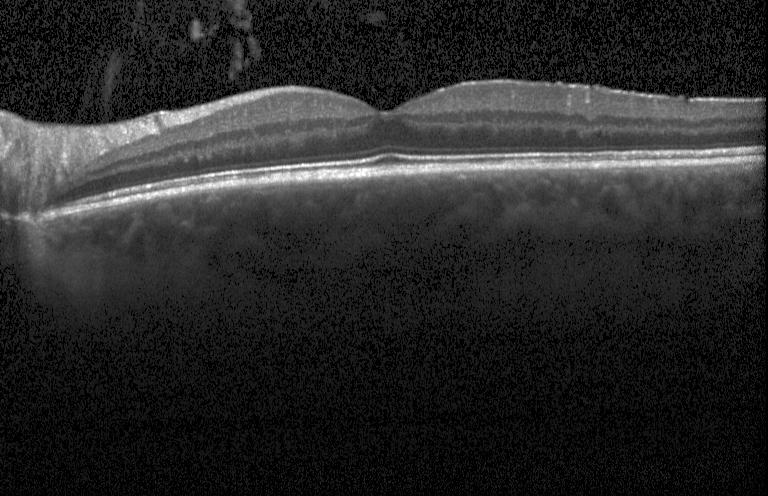 Optical coherence tomography B-scan — Dx: no evidence of choroidal neovascularization, diabetic macular edema, or drusen.